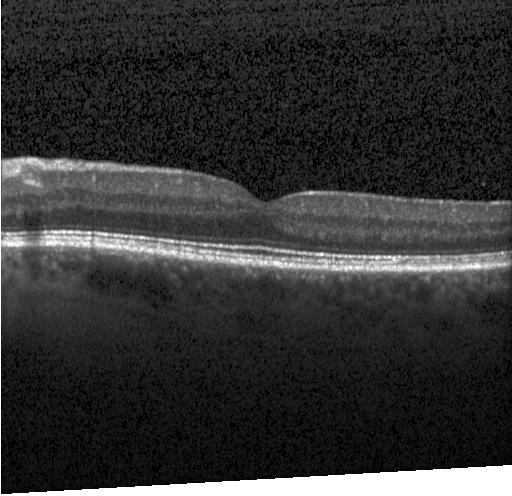 Optical coherence tomography B-scan. Spectral-domain OCT. Acquired on a Heidelberg Spectralis
Impression: neither choroidal neovascularization, diabetic macular edema, nor drusen.